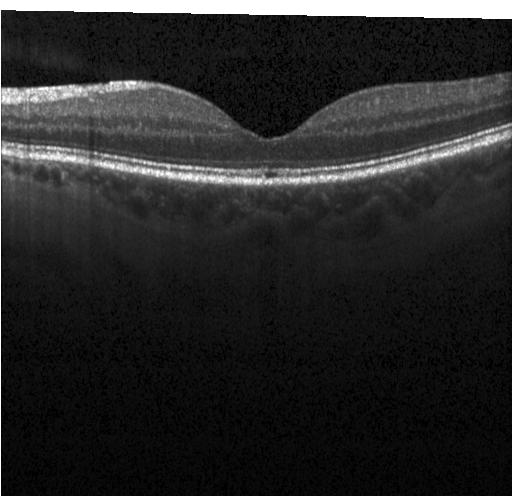
Finding: no choroidal neovascularization, no diabetic macular edema, and no drusen.